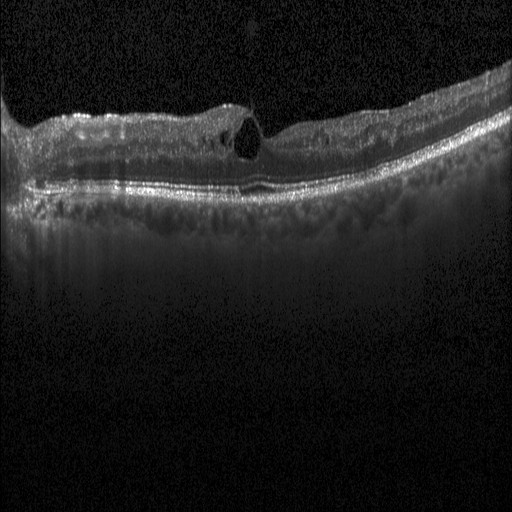
Optical coherence tomography B-scan · through the macula. Impression: diabetic macular edema.